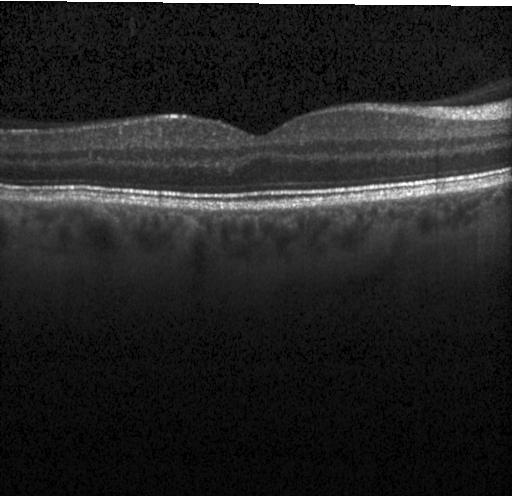
Spectral-domain optical coherence tomography. Through the macula. OCT line scan. Instrument: Heidelberg Spectralis
Diagnosis: neither choroidal neovascularization, diabetic macular edema, nor drusen.